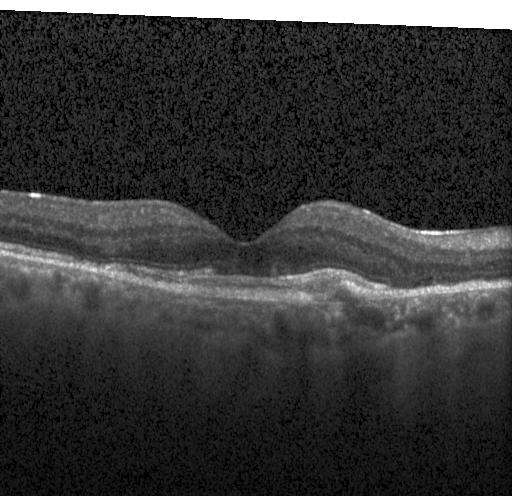 Heidelberg Spectralis OCT system. Horizontal scan through the fovea. Retinal OCT cross-section — This B-scan demonstrates a choroidal neovascular membrane.